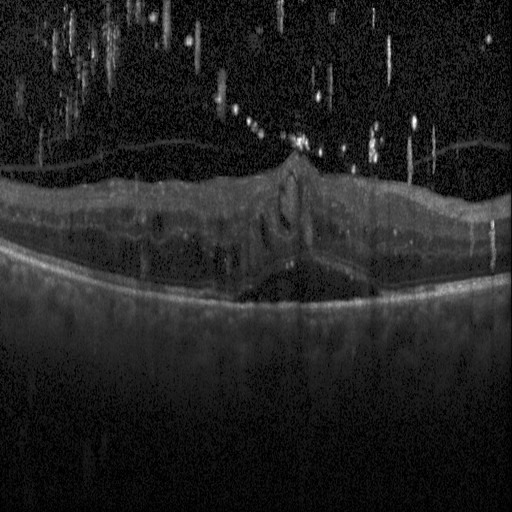
OCT B-scan, spectral-domain OCT, Heidelberg Spectralis. Diagnosis: diabetic macular edema (DME).